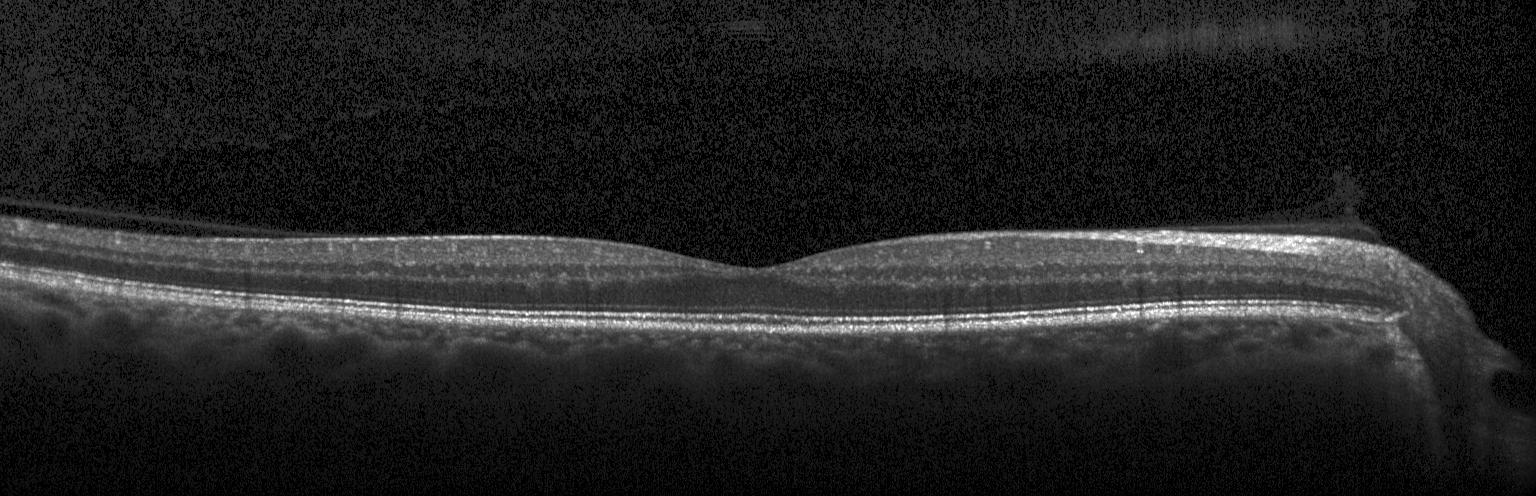

Heidelberg Spectralis, centered on the fovea, spectral-domain OCT, optical coherence tomography scan.
Finding: no choroidal neovascularization, diabetic macular edema, or drusen.